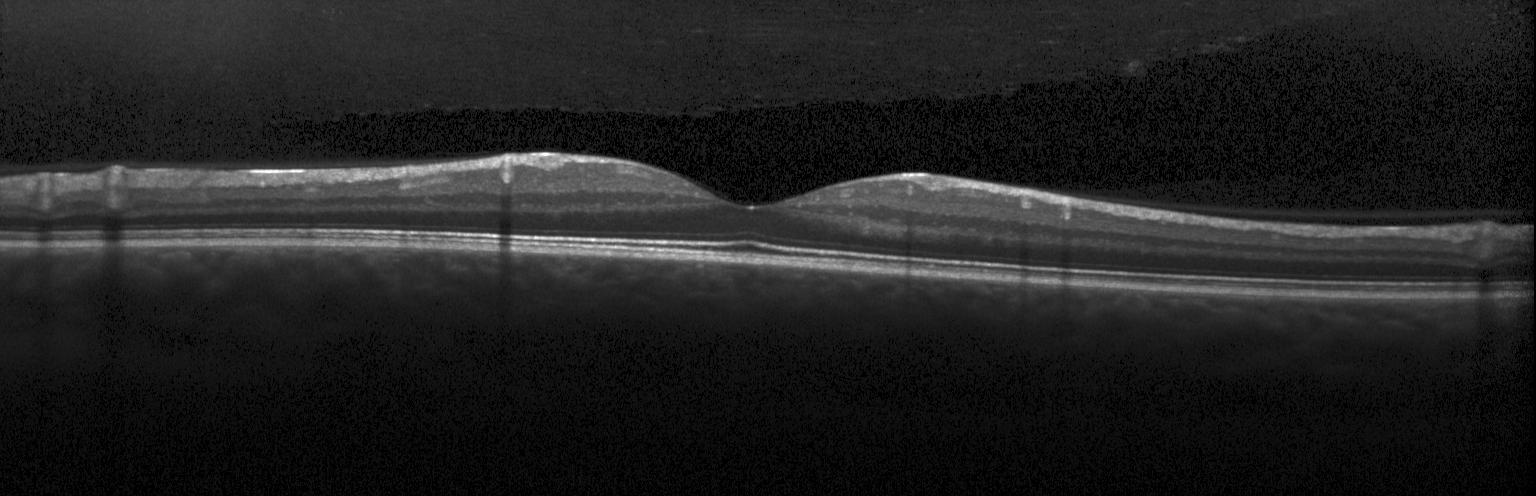 Optical coherence tomography B-scan. Assessment: neither CNV, DME, nor drusen.